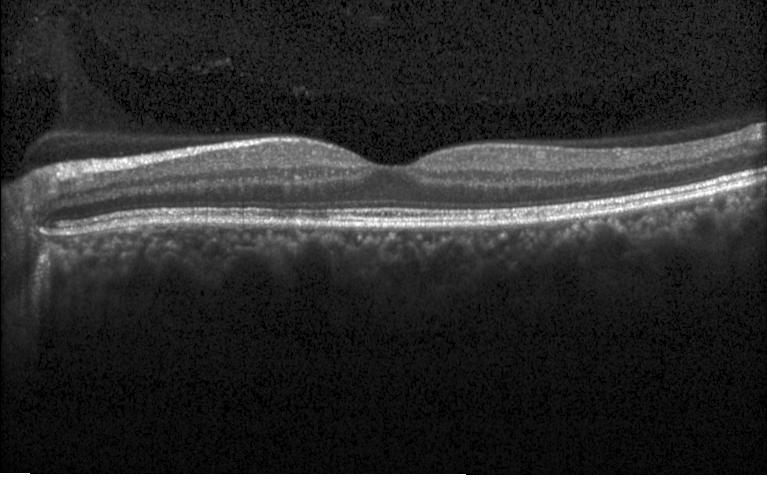 Spectral-domain optical coherence tomography, centered on the fovea, Heidelberg Spectralis OCT system, optical coherence tomography scan — Diagnosis: no choroidal neovascularization, no diabetic macular edema, and no drusen.